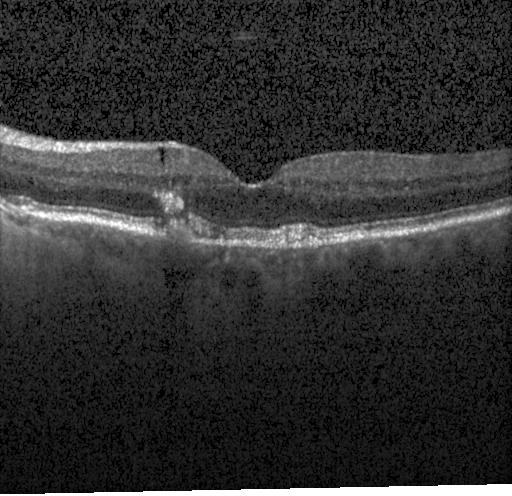 Finding: sub-RPE drusenoid deposits.